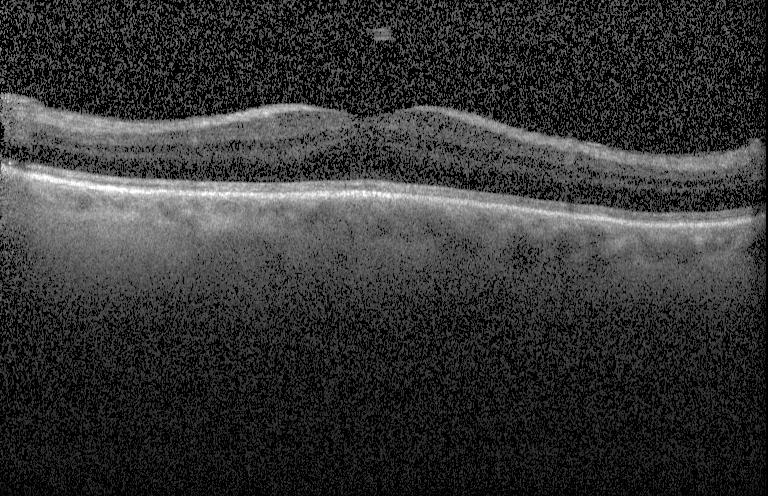
Diagnosis: neither CNV, DME, nor drusen.